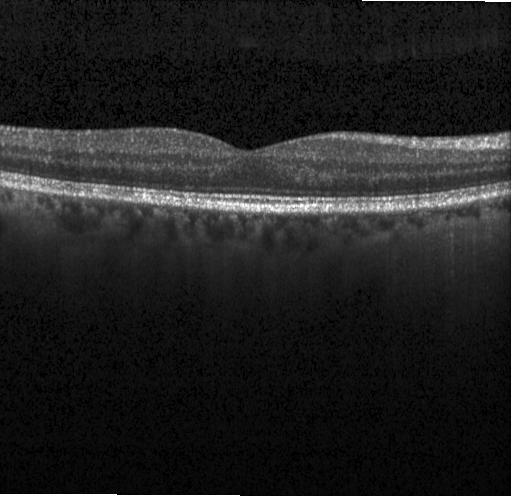
Through the macula · acquired on a Heidelberg Spectralis · spectral-domain optical coherence tomography · optical coherence tomography scan — Dx: no choroidal neovascularization, no diabetic macular edema, and no drusen.